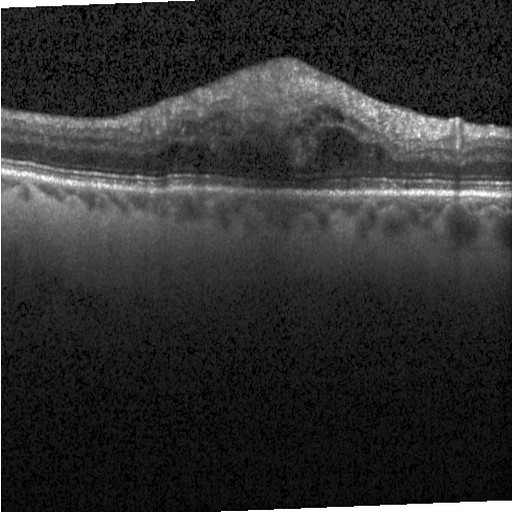 Through the macula · SD-OCT · OCT line scan · Heidelberg Spectralis OCT system.
This B-scan demonstrates DME.